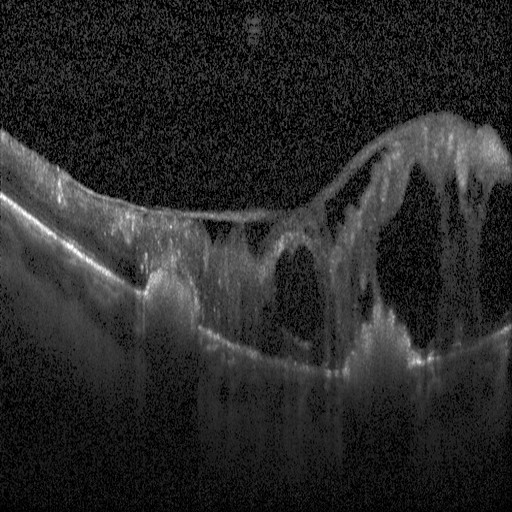

Optical coherence tomography scan; SD-OCT.
Impression: diabetic macular edema.